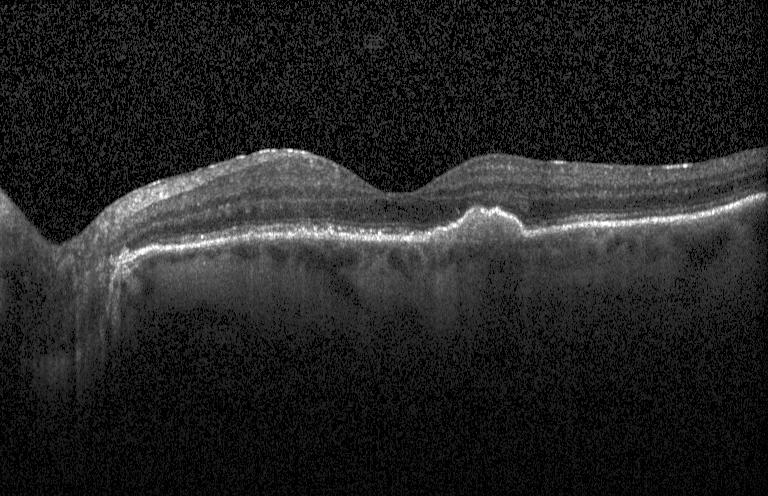
Instrument: Heidelberg Spectralis, retinal OCT B-scan, horizontal scan through the fovea, SD-OCT. Dx: CNV.